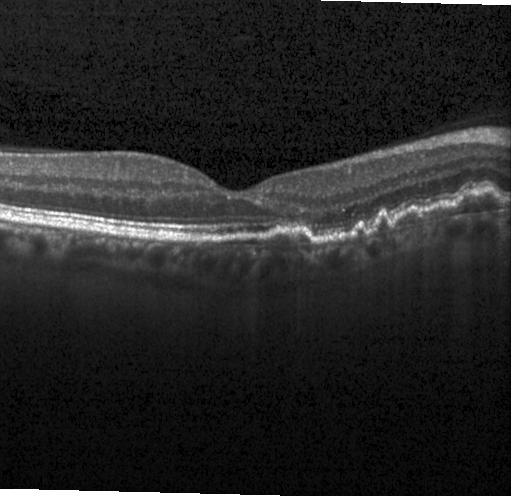

OCT line scan, macular scan
This B-scan demonstrates a choroidal neovascular membrane.